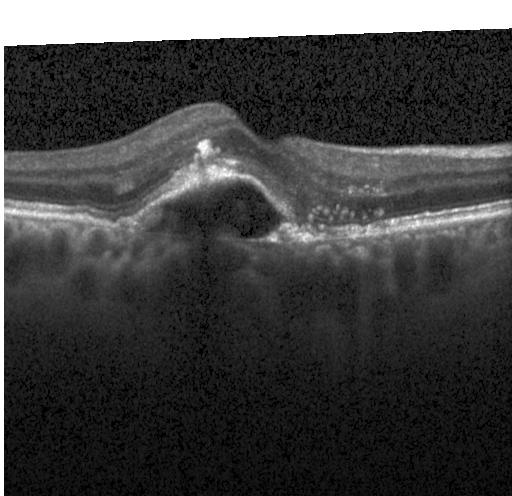 OCT finding: a choroidal neovascular membrane.